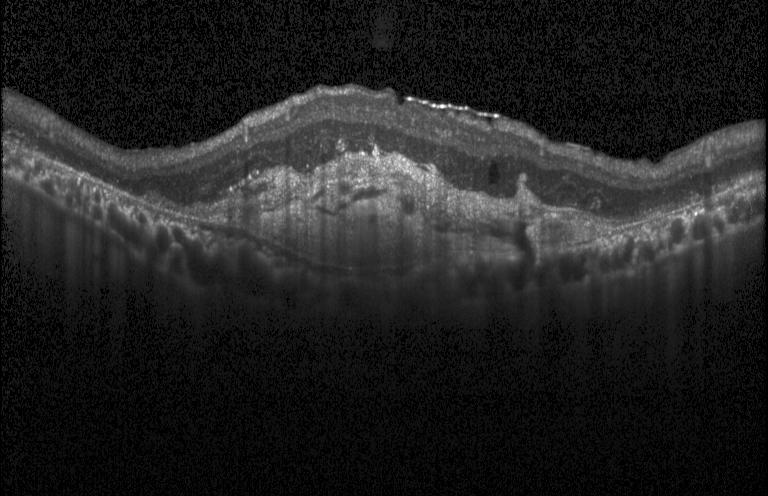 Spectral-domain OCT; OCT line scan; acquired on a Heidelberg Spectralis — This B-scan demonstrates a choroidal neovascular membrane.